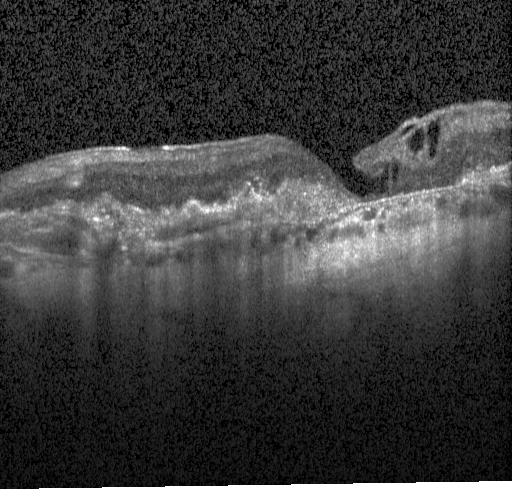 SD-OCT, retinal OCT B-scan
Impression: a choroidal neovascular membrane.